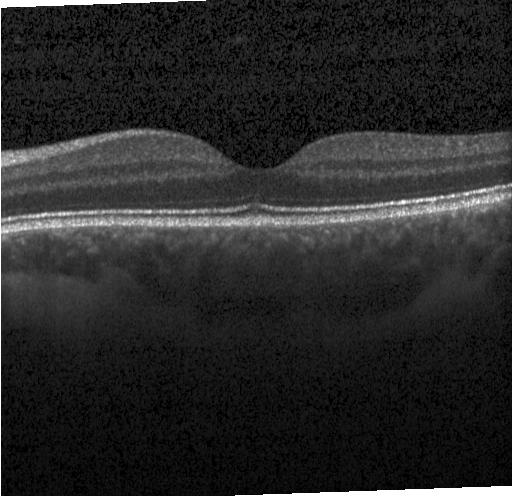

Optical coherence tomography B-scan. Impression: neither choroidal neovascularization, diabetic macular edema, nor drusen.